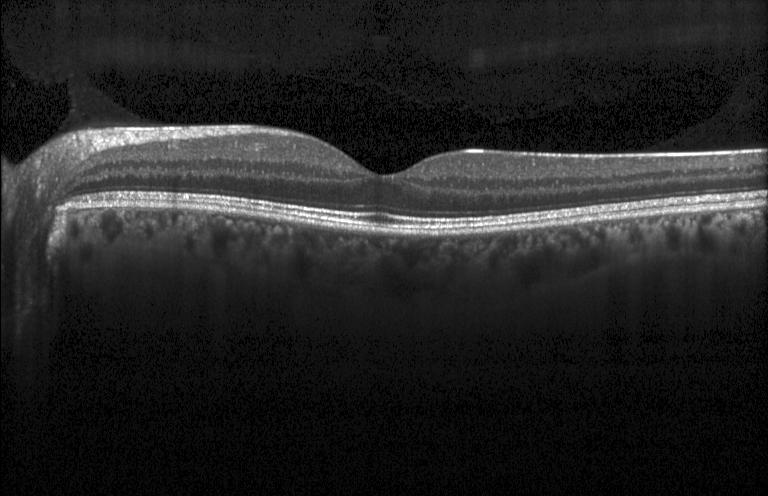 Macular scan; spectral-domain OCT; OCT B-scan — No choroidal neovascularization, no diabetic macular edema, and no drusen.